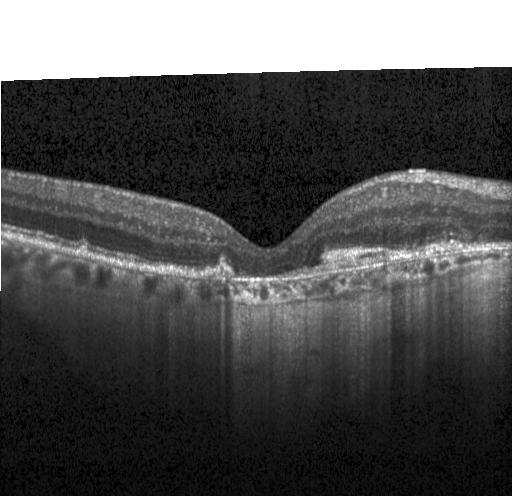

Macular scan; spectral-domain optical coherence tomography; optical coherence tomography scan; acquired on a Heidelberg Spectralis — Finding: a choroidal neovascular membrane.